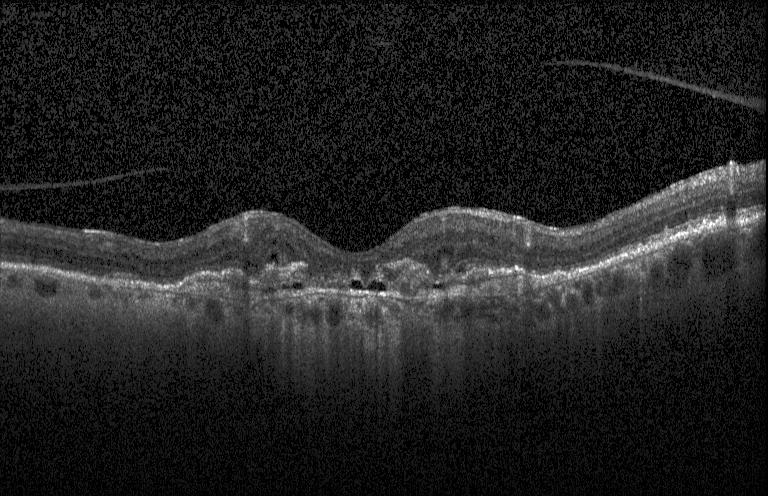
Retinal OCT B-scan; through the macula; SD-OCT. Assessment: a choroidal neovascular membrane.